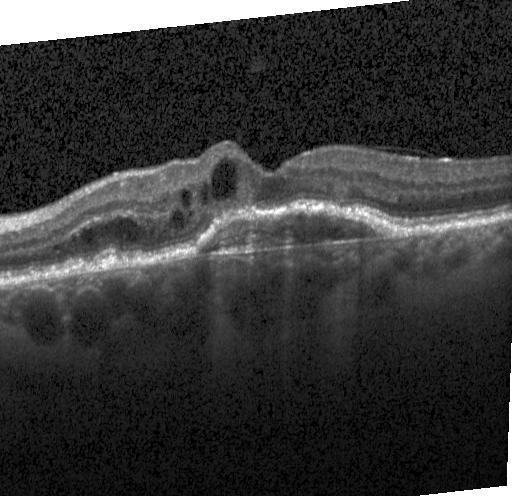

Impression: a choroidal neovascular membrane.